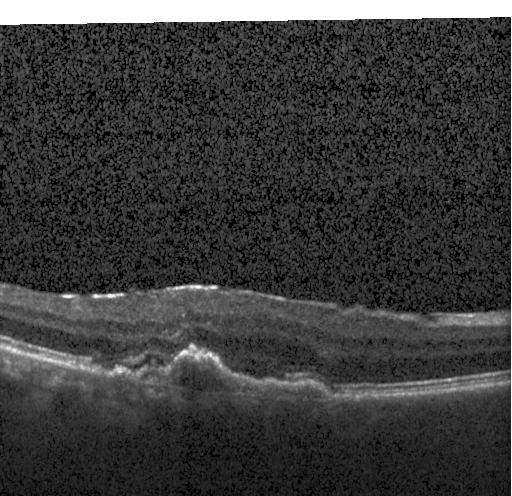 Retinal OCT cross-section · through the macula — Finding: CNV.